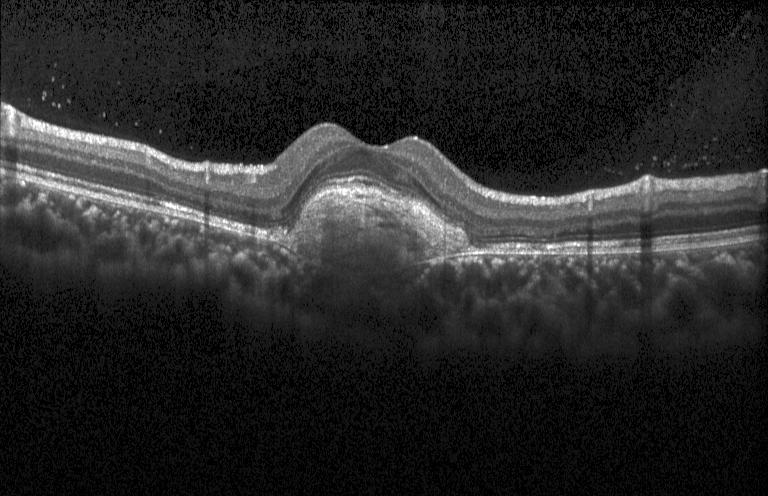 SD-OCT. OCT B-scan. Acquired on a Heidelberg Spectralis.
The scan shows a choroidal neovascular membrane.